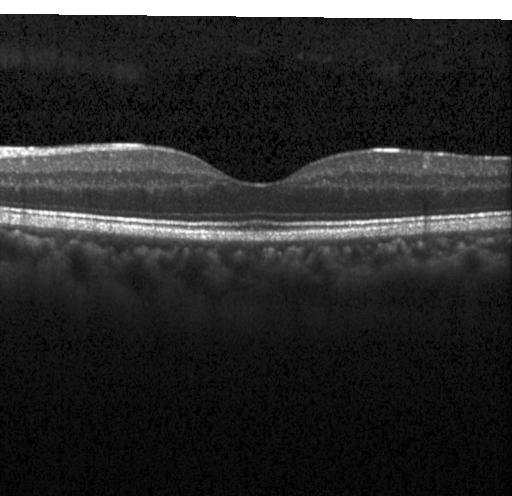

Diagnosis: neither CNV, DME, nor drusen.